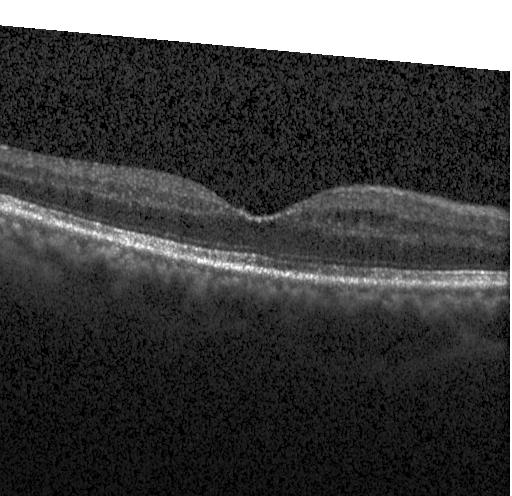
SD-OCT. Retinal OCT B-scan. Heidelberg Spectralis OCT system.
Finding: no choroidal neovascularization, no diabetic macular edema, and no drusen.